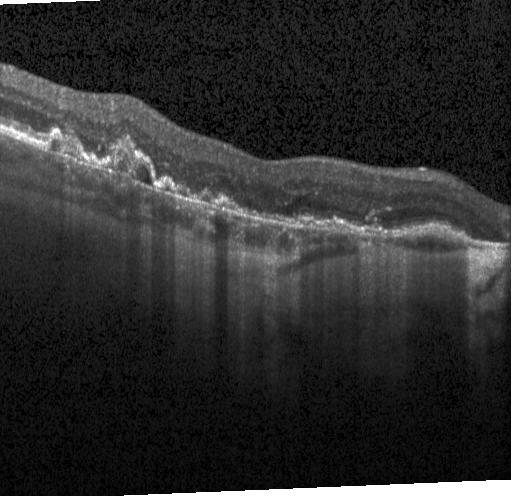

Instrument: Heidelberg Spectralis; OCT B-scan. This B-scan demonstrates CNV.